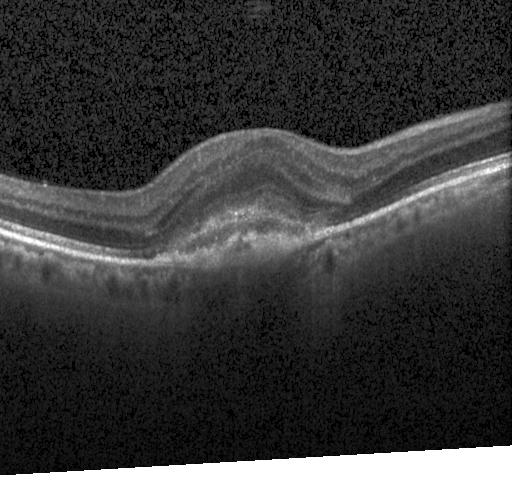
Macular scan. Retinal OCT cross-section. Heidelberg Spectralis. Finding: a choroidal neovascular membrane.